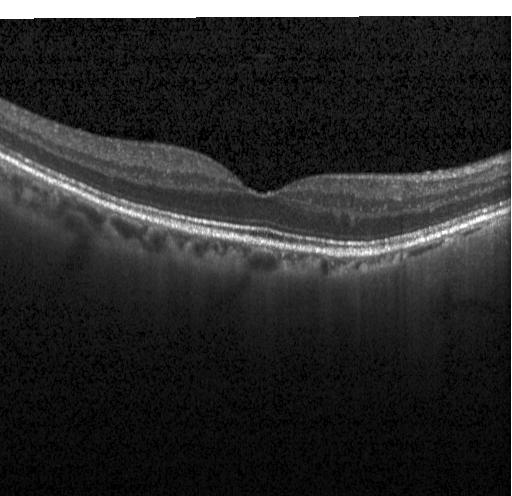

Acquired on a Heidelberg Spectralis · horizontal scan through the fovea · OCT B-scan. Dx: no choroidal neovascularization, diabetic macular edema, or drusen.